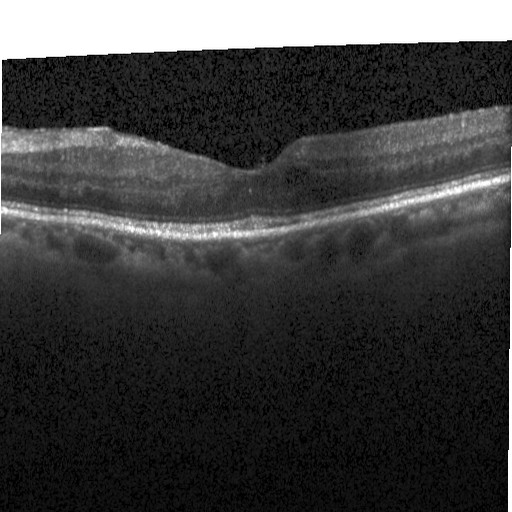

This B-scan demonstrates DME.